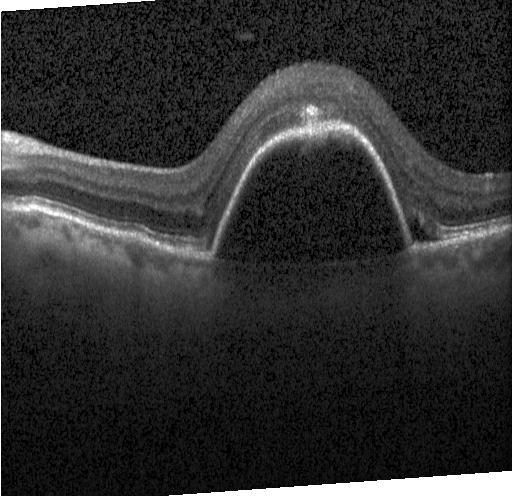

Optical coherence tomography scan, horizontal scan through the fovea, acquired on a Heidelberg Spectralis, spectral-domain OCT. Dx: a choroidal neovascular membrane.